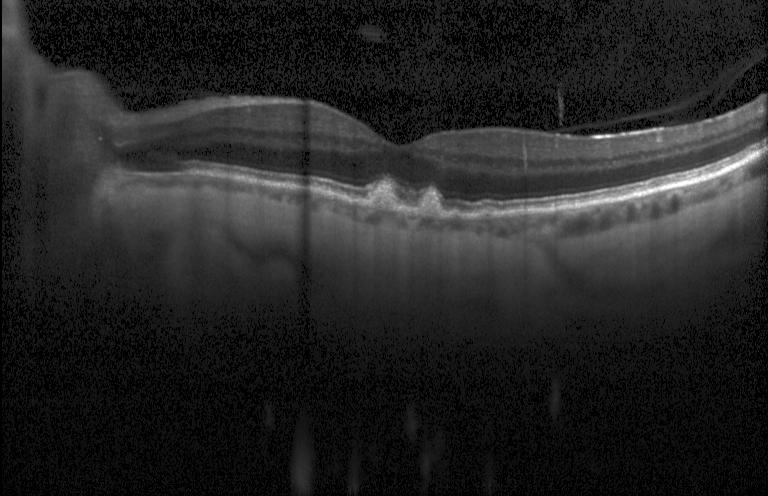

Heidelberg Spectralis, optical coherence tomography B-scan
Diagnosis: sub-RPE drusenoid deposits.